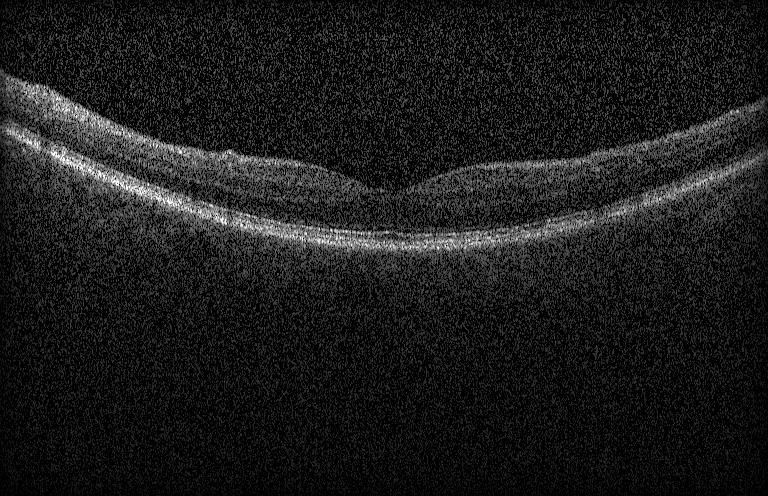 Impression: no evidence of choroidal neovascularization, diabetic macular edema, or drusen.